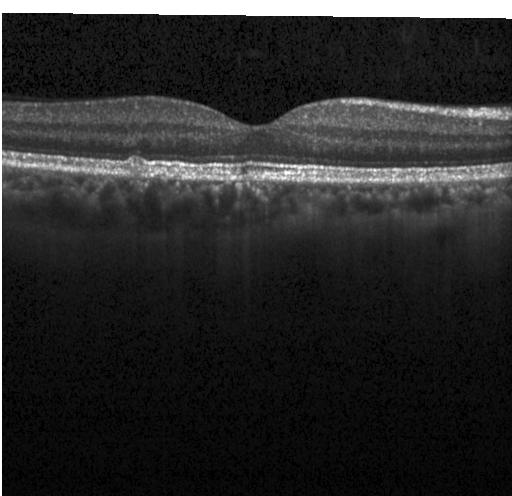
Instrument: Heidelberg Spectralis, horizontal scan through the fovea, SD-OCT, optical coherence tomography scan — The scan shows multiple drusen.